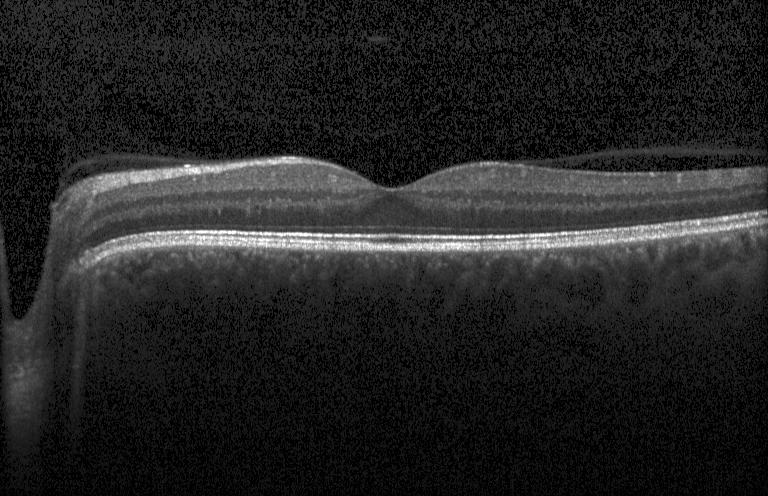 Heidelberg Spectralis OCT system; SD-OCT; centered on the fovea; optical coherence tomography scan
Impression: no choroidal neovascularization, no diabetic macular edema, and no drusen.